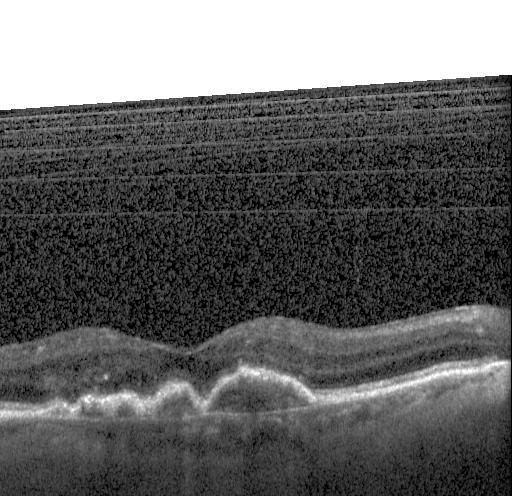

Retinal OCT B-scan. Impression: CNV.